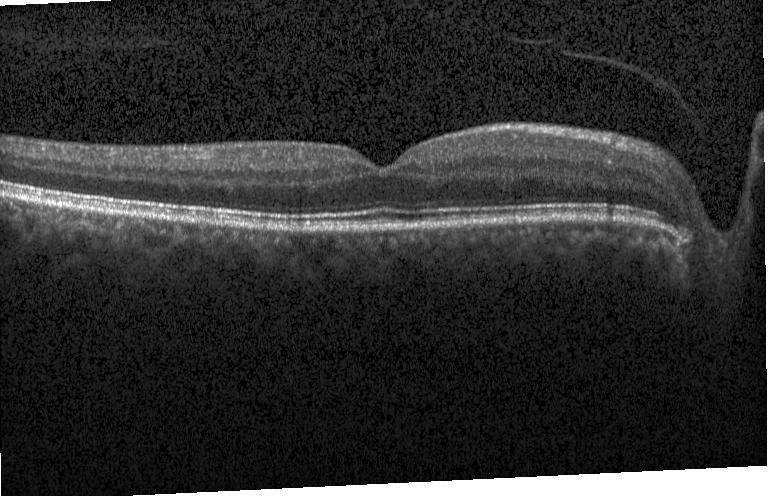
OCT line scan · macular scan · SD-OCT · instrument: Heidelberg Spectralis.
Assessment: no choroidal neovascularization, no diabetic macular edema, and no drusen.